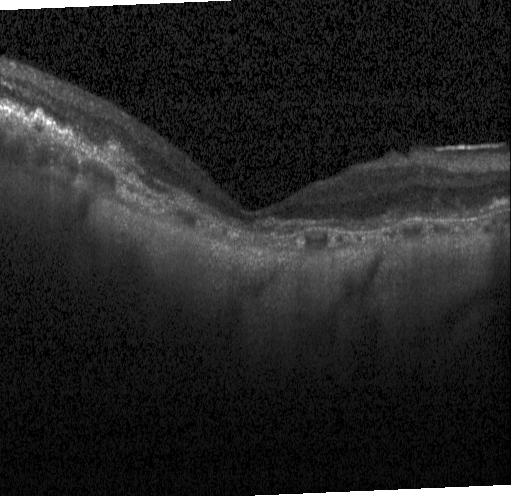
Acquired on a Heidelberg Spectralis; SD-OCT; optical coherence tomography B-scan.
Dx: a choroidal neovascular membrane.